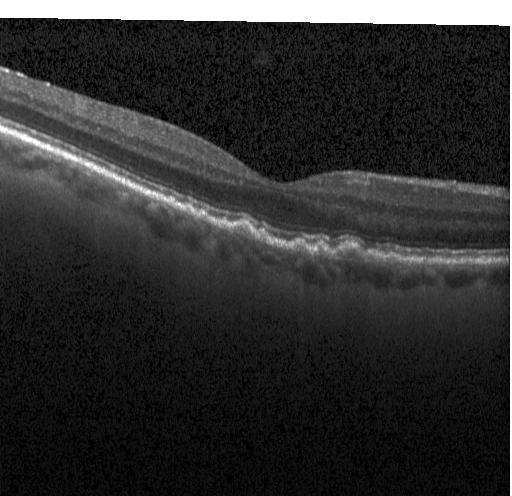
OCT finding: sub-RPE drusenoid deposits.